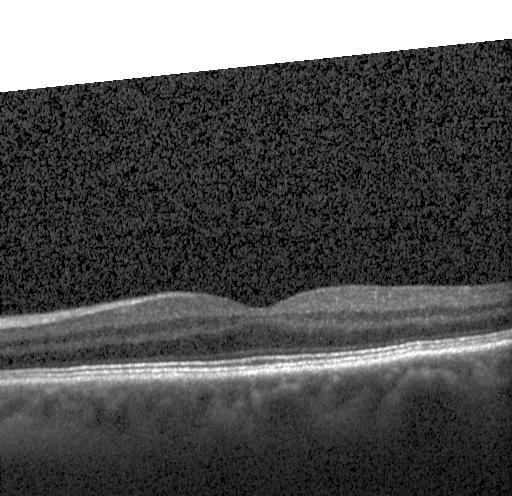
Through the macula, spectral-domain OCT, acquired on a Heidelberg Spectralis, retinal OCT B-scan — Diagnosis: no evidence of CNV, DME, or drusen.